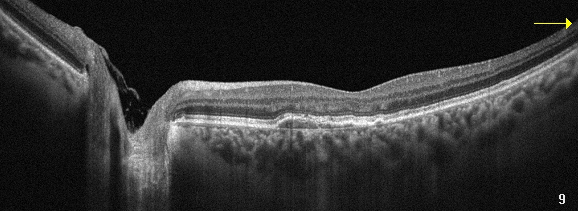
Finding: age-related macular degeneration.